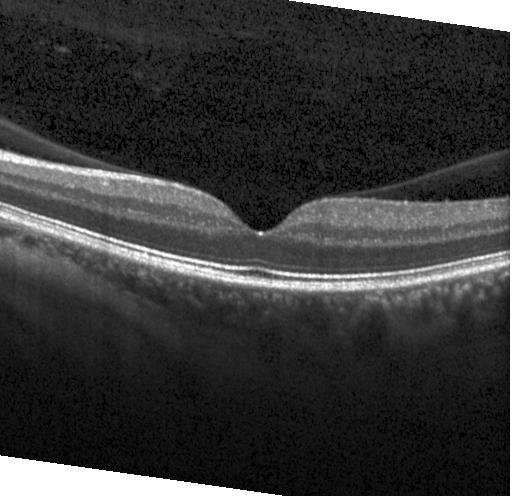
OCT line scan; Heidelberg Spectralis OCT system.
Diagnosis: no CNV, no DME, and no drusen.